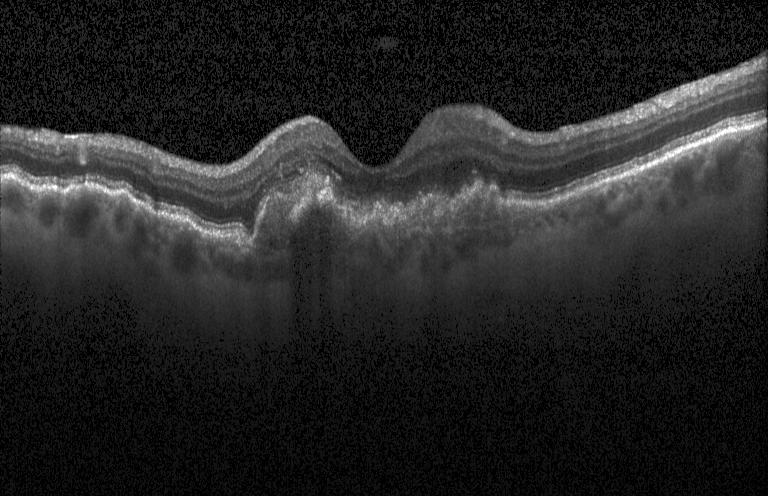 Optical coherence tomography scan · SD-OCT · Heidelberg Spectralis. This B-scan demonstrates choroidal neovascularization.